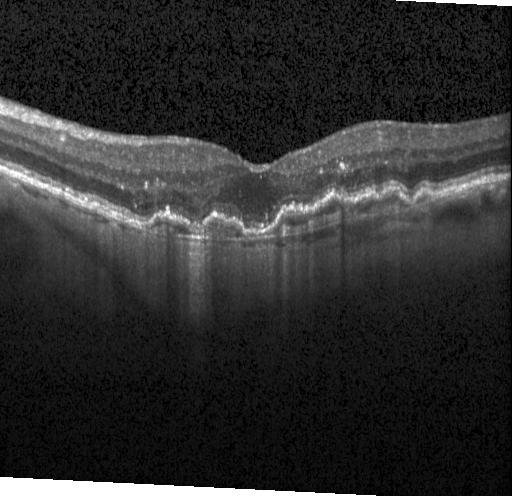 Horizontal scan through the fovea, spectral-domain optical coherence tomography, OCT B-scan, instrument: Heidelberg Spectralis
A choroidal neovascular membrane.